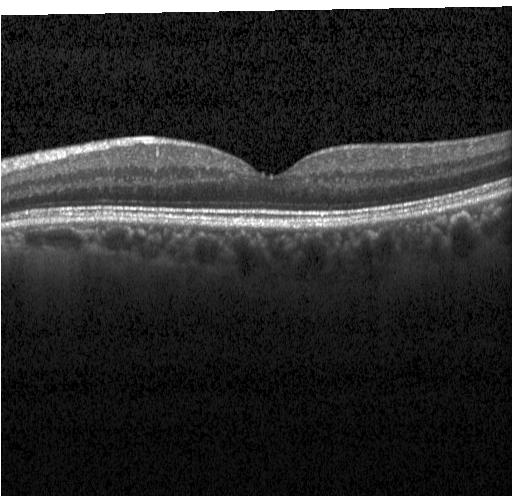 Optical coherence tomography B-scan; spectral-domain OCT; fovea-centered.
This B-scan demonstrates neither CNV, DME, nor drusen.